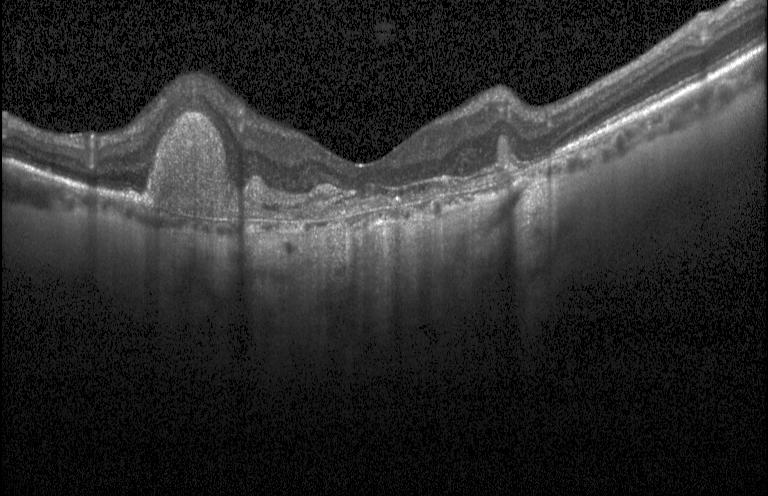 Retinal OCT cross-section, spectral-domain optical coherence tomography, centered on the fovea, instrument: Heidelberg Spectralis.
Assessment: CNV.